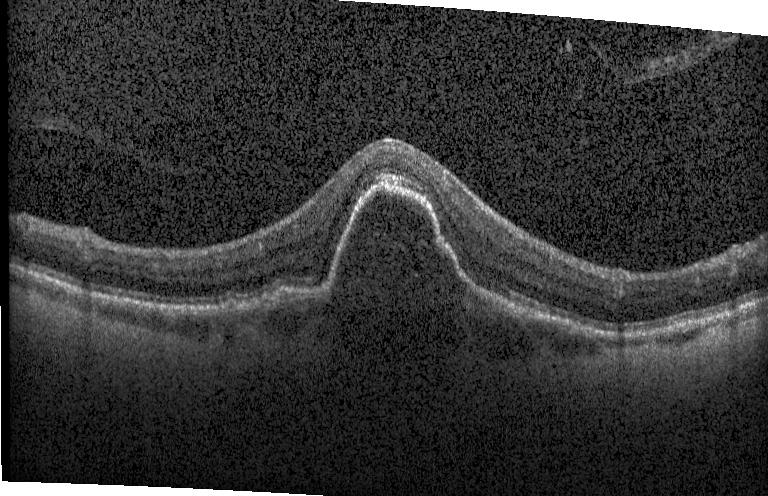

Finding: CNV.